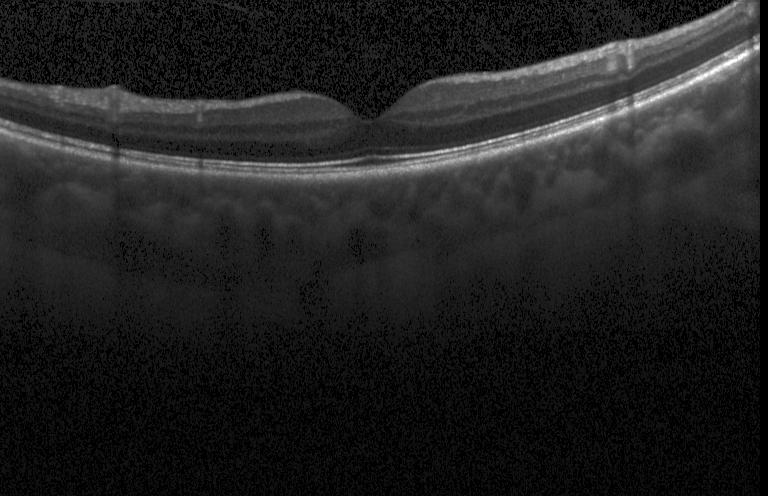
Retinal OCT B-scan.
Macular OCT: neither choroidal neovascularization, diabetic macular edema, nor drusen.